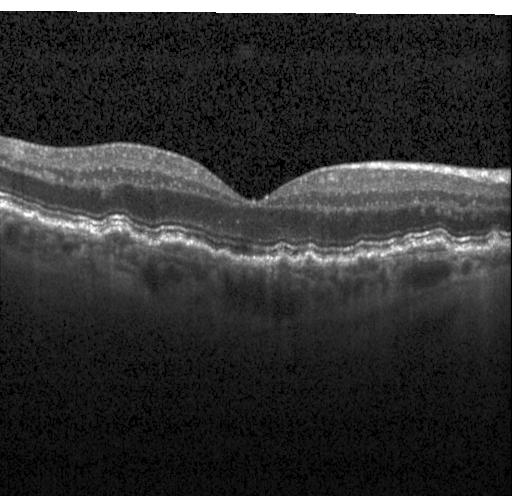

Optical coherence tomography B-scan
Dx: multiple drusen.